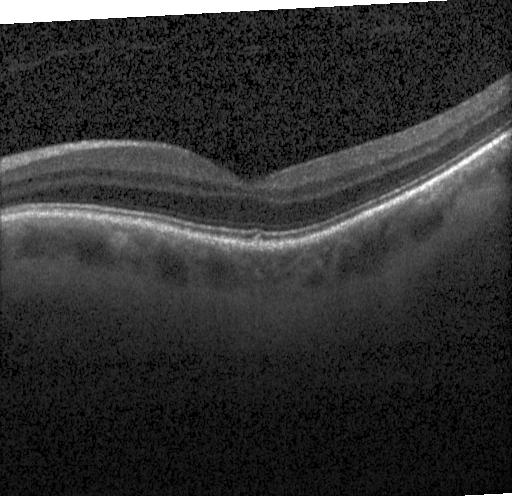
Impression: neither CNV, DME, nor drusen.